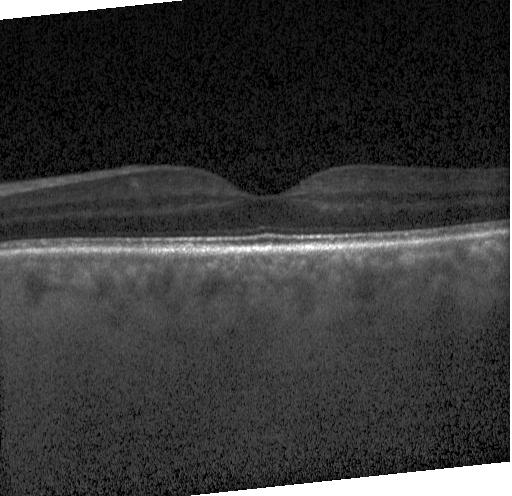
Retinal OCT cross-section; centered on the fovea; instrument: Heidelberg Spectralis; spectral-domain optical coherence tomography.
Impression: no CNV, DME, or drusen.